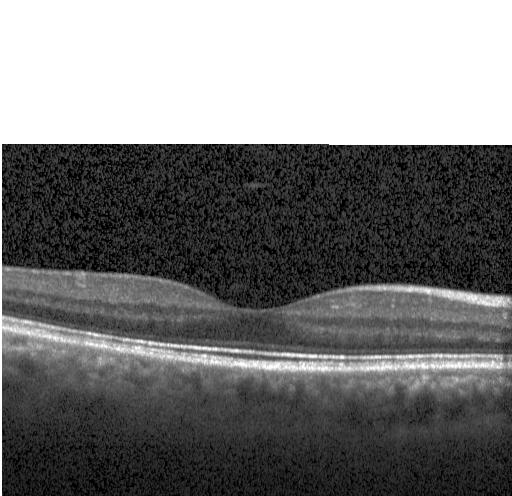

Retinal OCT cross-section. Diagnosis: neither choroidal neovascularization, diabetic macular edema, nor drusen.